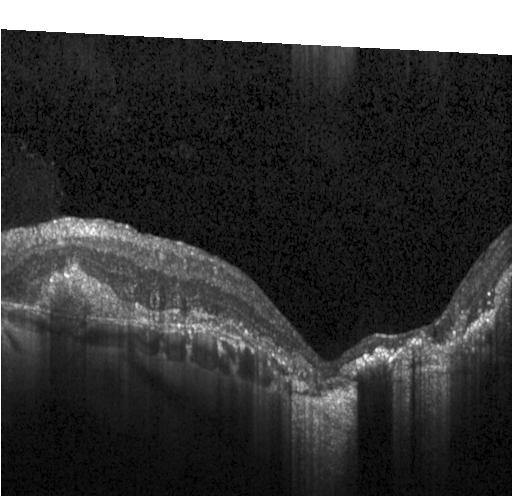

Spectral-domain OCT B-scan: a choroidal neovascular membrane.